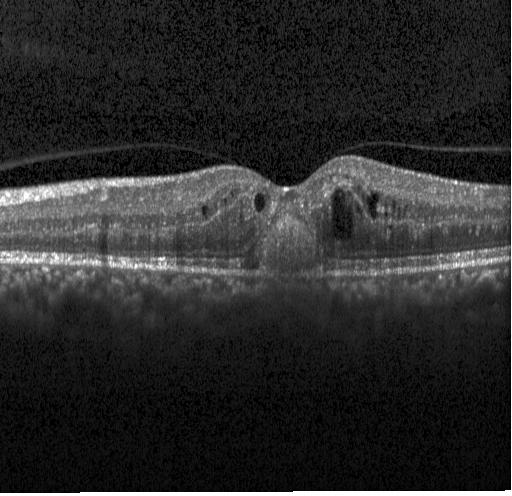
OCT B-scan.
Finding: CNV.